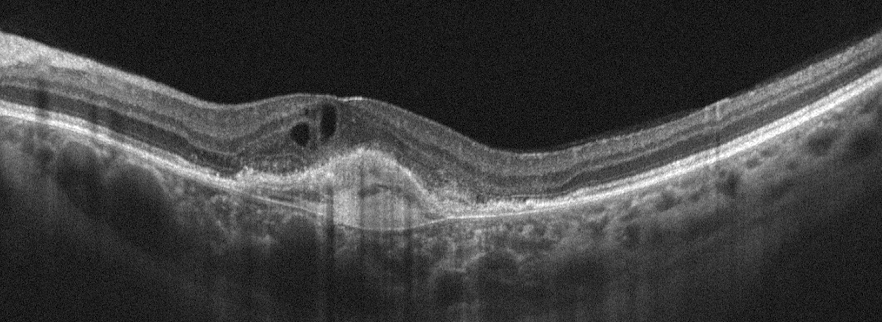
Optical coherence tomography scan. OS
Macular OCT: AMD.